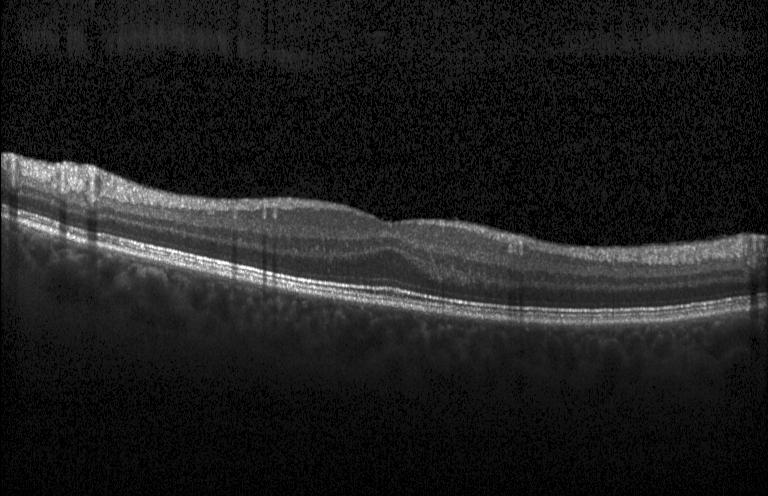
The scan shows neither choroidal neovascularization, diabetic macular edema, nor drusen.